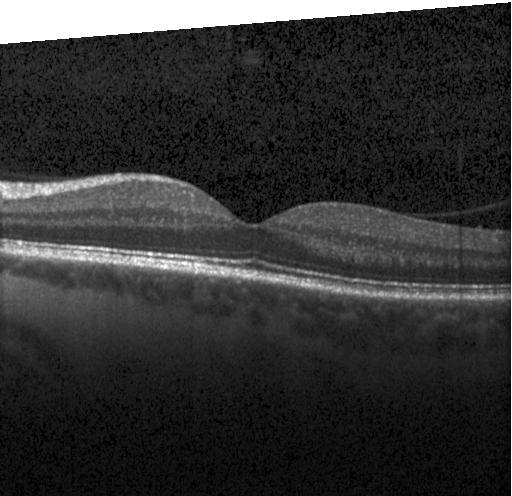

Optical coherence tomography scan, acquired on a Heidelberg Spectralis, macular scan — This B-scan demonstrates no evidence of choroidal neovascularization, diabetic macular edema, or drusen.